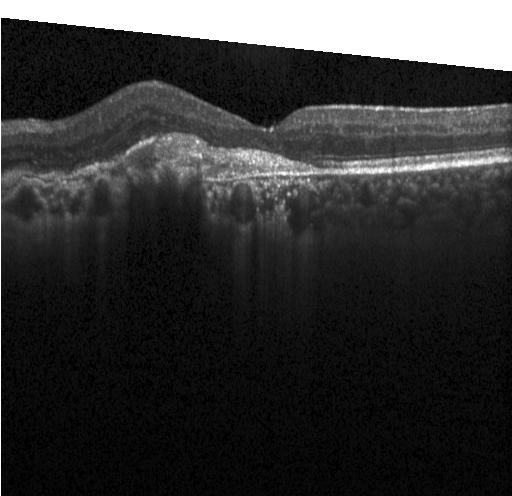

Through the macula; instrument: Heidelberg Spectralis; optical coherence tomography scan
Dx: choroidal neovascularization.